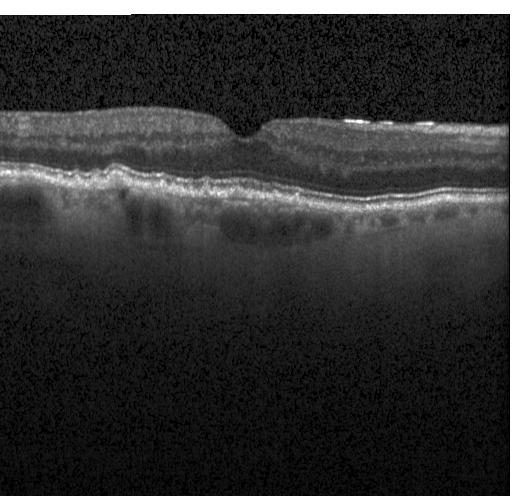 Optical coherence tomography scan; spectral-domain optical coherence tomography; Heidelberg Spectralis
This B-scan demonstrates sub-RPE drusenoid deposits.